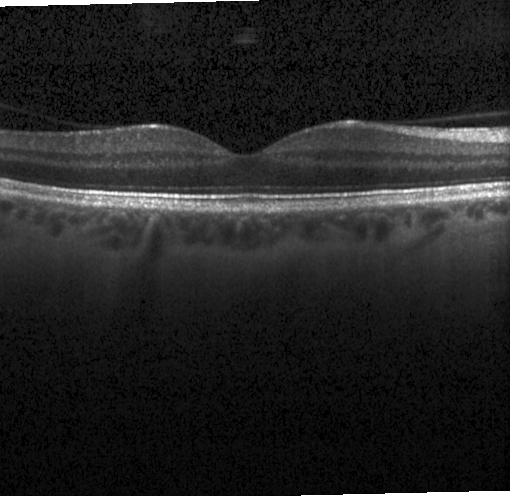

OCT finding: no choroidal neovascularization, diabetic macular edema, or drusen.